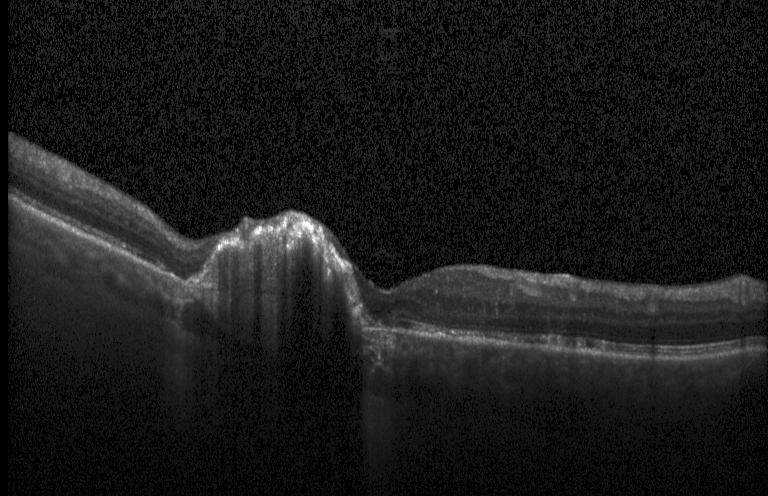

Spectral-domain OCT. Acquired on a Heidelberg Spectralis. Horizontal scan through the fovea. Retinal OCT cross-section
Diagnosis: CNV.